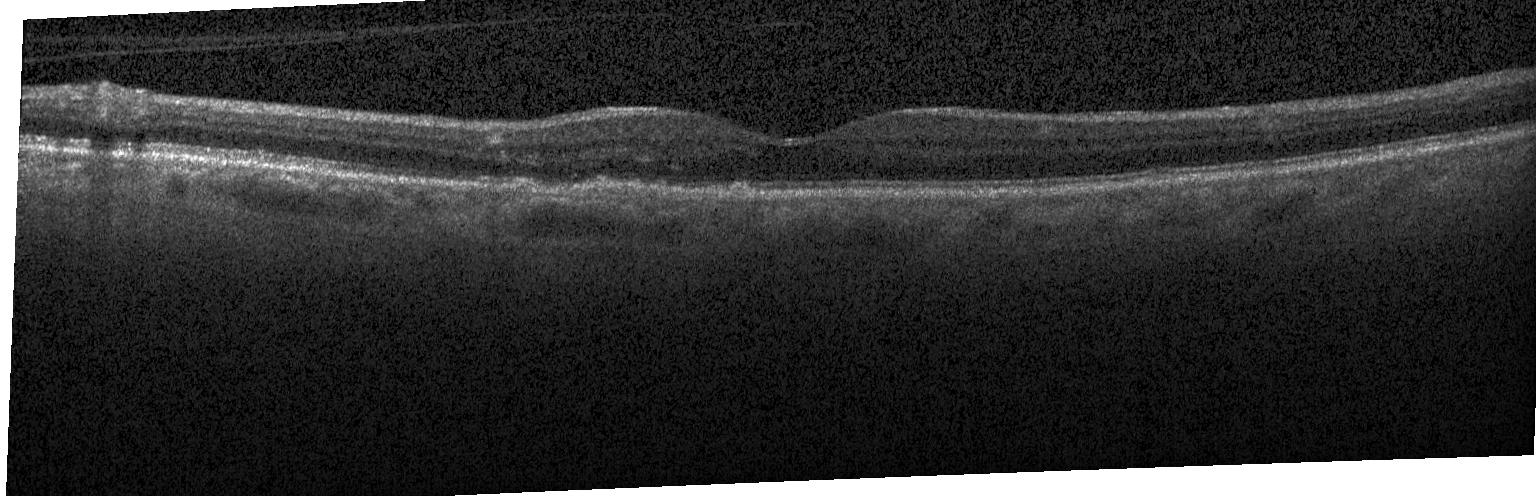
OCT B-scan, spectral-domain optical coherence tomography.
Impression: sub-RPE drusenoid deposits.